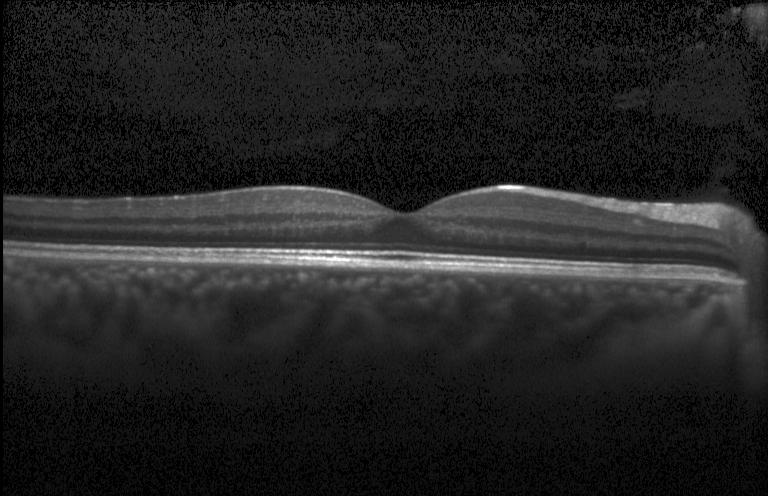
Acquired on a Heidelberg Spectralis · retinal OCT B-scan — Assessment: no evidence of choroidal neovascularization, diabetic macular edema, or drusen.